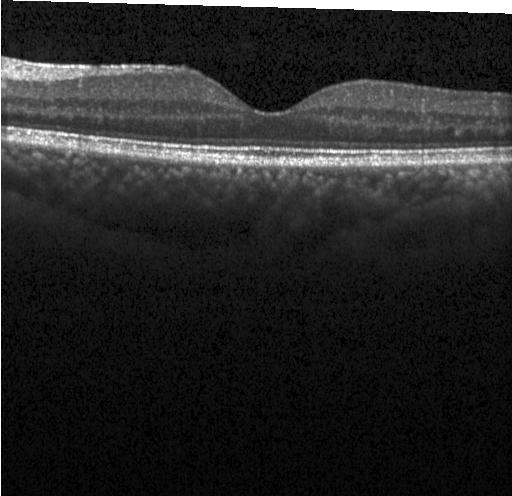

No CNV, DME, or drusen.